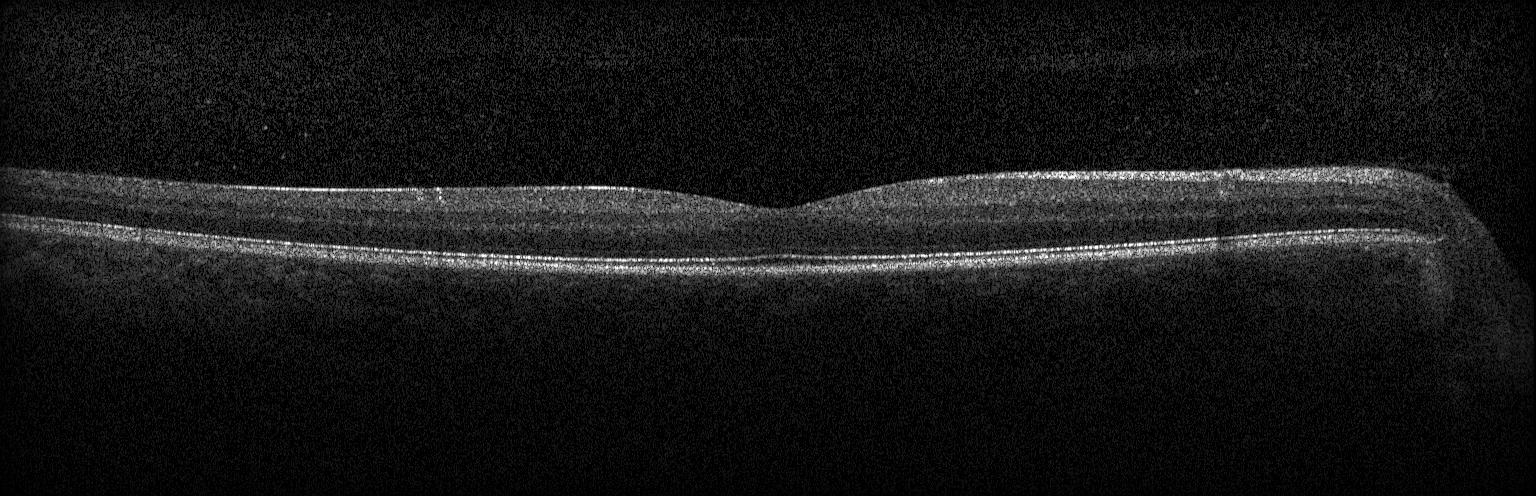
Finding: no evidence of choroidal neovascularization, diabetic macular edema, or drusen.